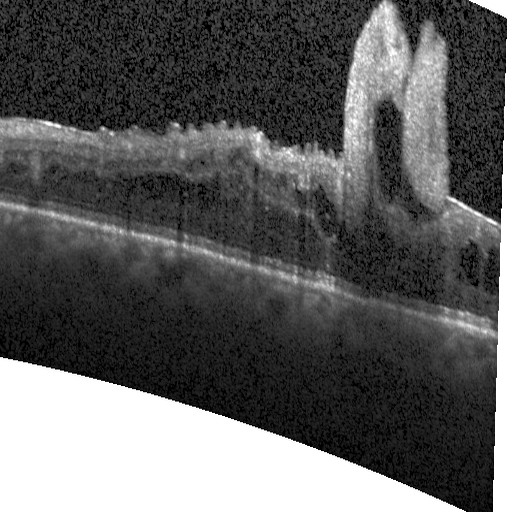 Optical coherence tomography scan. Impression: diabetic macular edema.